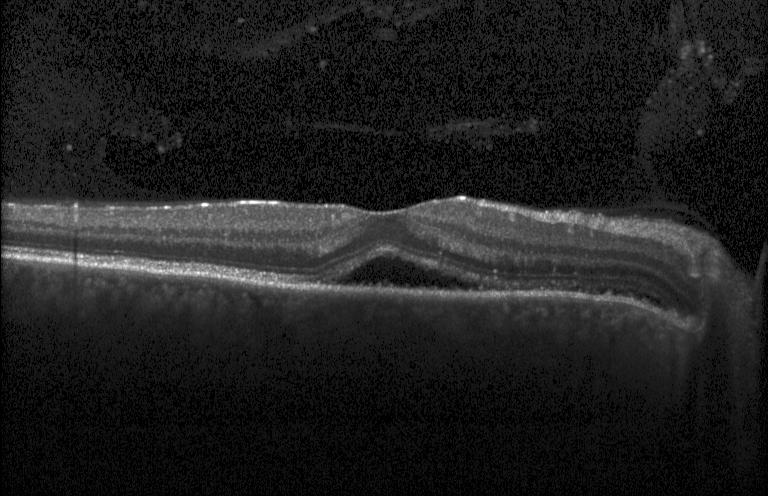 Acquired on a Heidelberg Spectralis, spectral-domain optical coherence tomography, through the macula, optical coherence tomography B-scan — OCT finding: choroidal neovascularization.